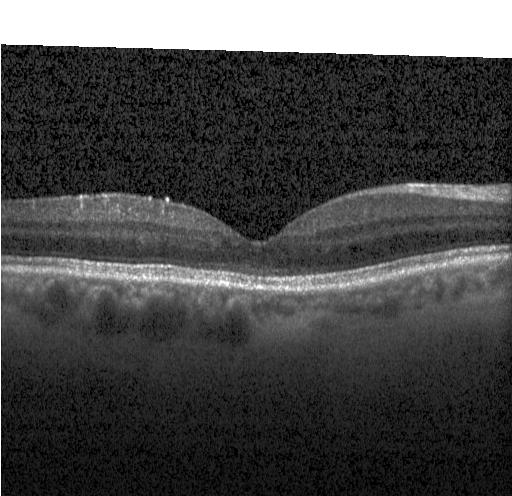 Optical coherence tomography B-scan · through the macula — The scan shows neither choroidal neovascularization, diabetic macular edema, nor drusen.